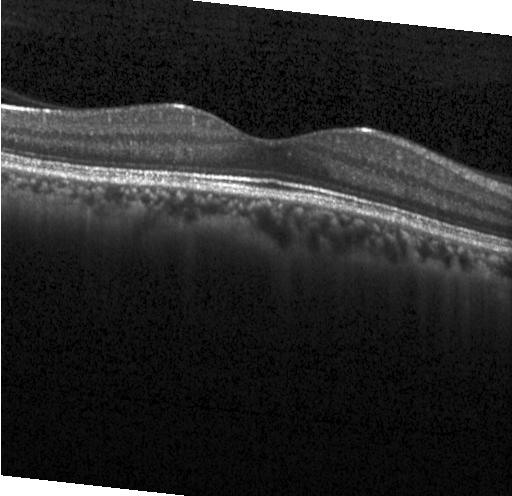
Retinal OCT cross-section · horizontal scan through the fovea · instrument: Heidelberg Spectralis
Dx: neither choroidal neovascularization, diabetic macular edema, nor drusen.